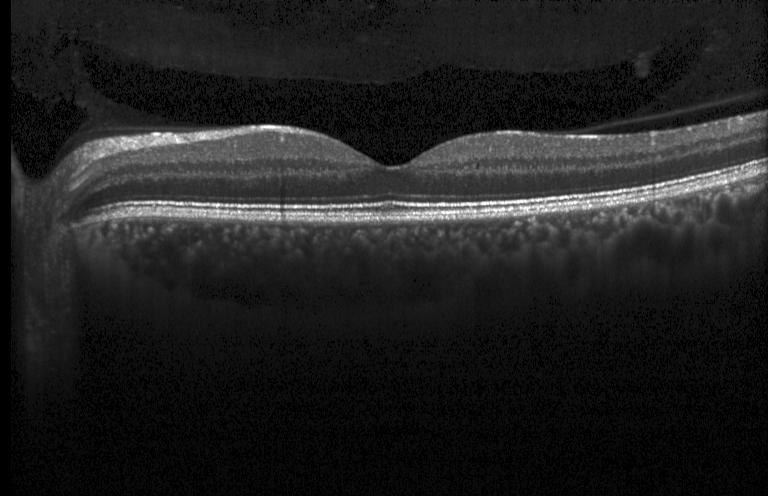

Macular scan · Heidelberg Spectralis · optical coherence tomography B-scan.
No CNV, DME, or drusen.